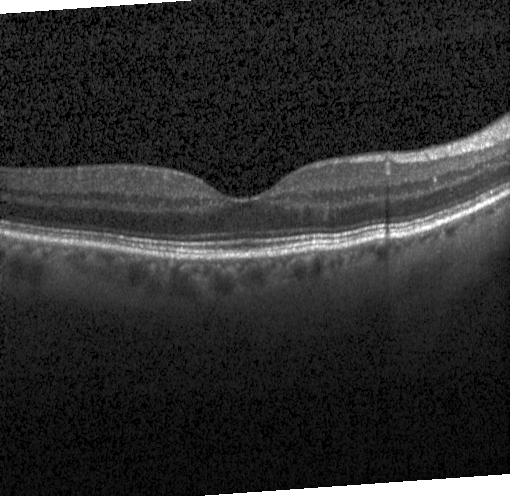

SD-OCT; acquired on a Heidelberg Spectralis; retinal OCT B-scan
Assessment: no evidence of choroidal neovascularization, diabetic macular edema, or drusen.